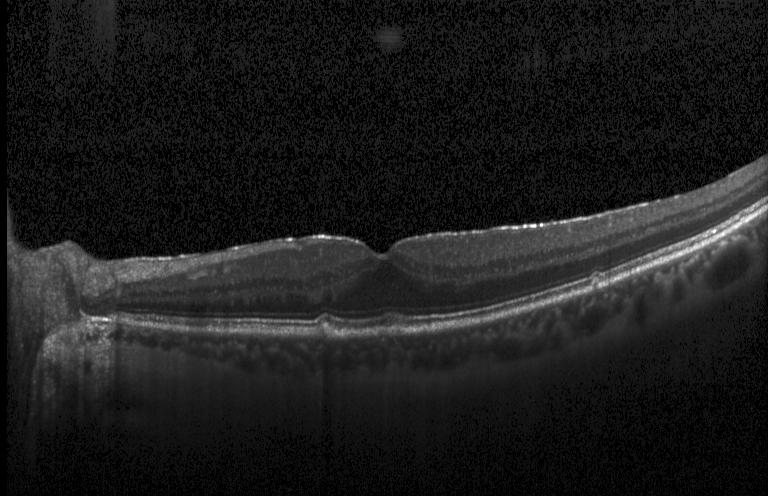

Horizontal scan through the fovea. Heidelberg Spectralis OCT system. OCT line scan. Spectral-domain OCT. Macular OCT: multiple drusen.